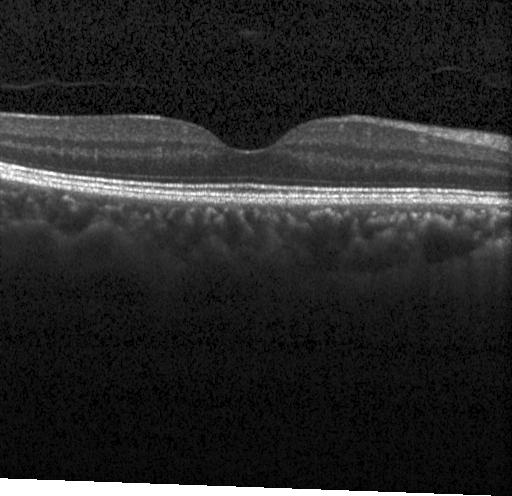

The scan shows no choroidal neovascularization, no diabetic macular edema, and no drusen.